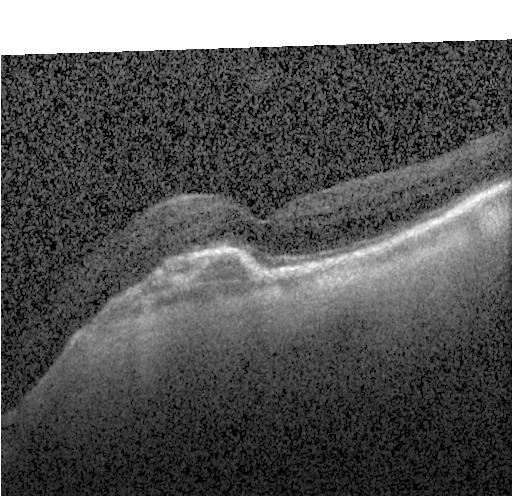

OCT B-scan; spectral-domain OCT.
Macular OCT: a choroidal neovascular membrane.